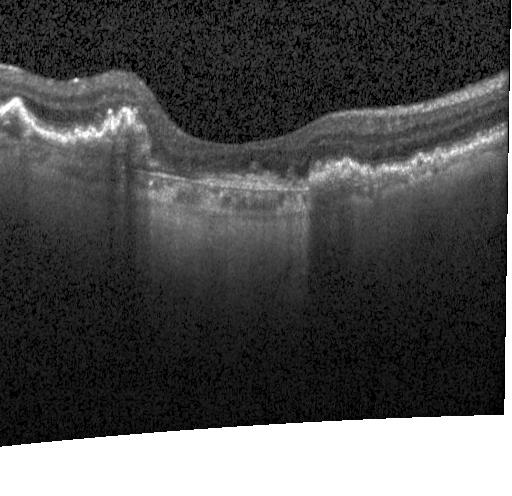
Acquired on a Heidelberg Spectralis. Retinal OCT cross-section. Spectral-domain optical coherence tomography. Through the macula. Impression: CNV.